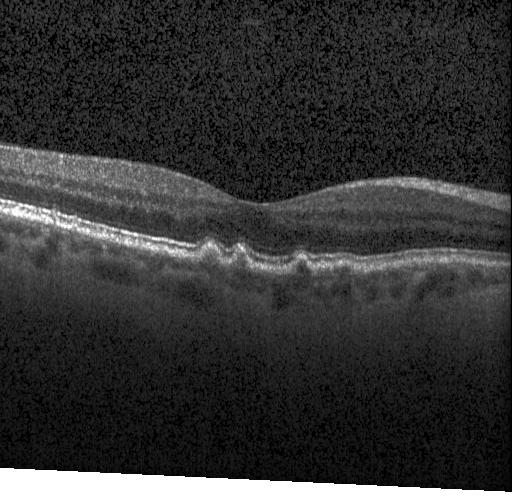 Acquired on a Heidelberg Spectralis; spectral-domain optical coherence tomography; fovea-centered; retinal OCT B-scan. Impression: drusen.